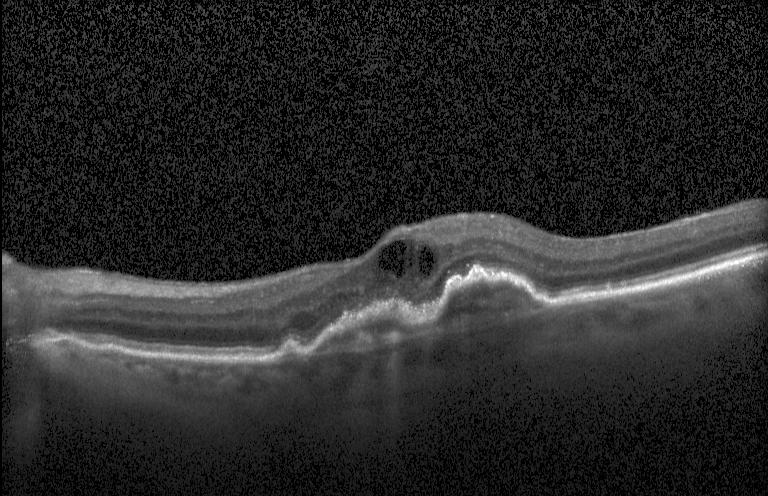

Heidelberg Spectralis OCT system · fovea-centered · optical coherence tomography B-scan · SD-OCT
Impression: choroidal neovascularization.